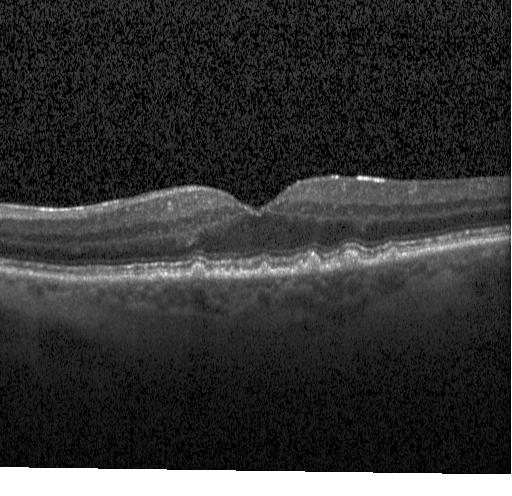 Heidelberg Spectralis, retinal OCT cross-section.
OCT finding: sub-RPE drusenoid deposits.